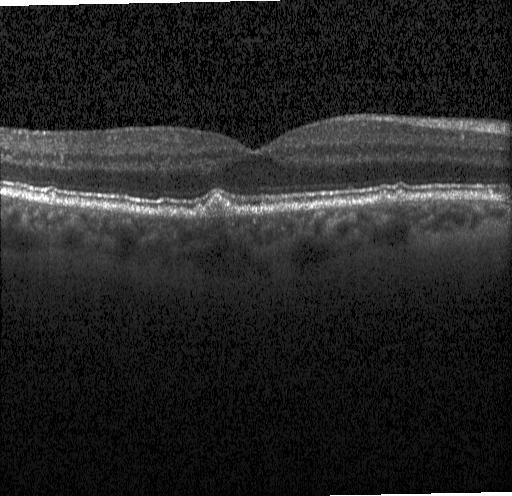
Spectral-domain OCT B-scan: sub-RPE drusenoid deposits.